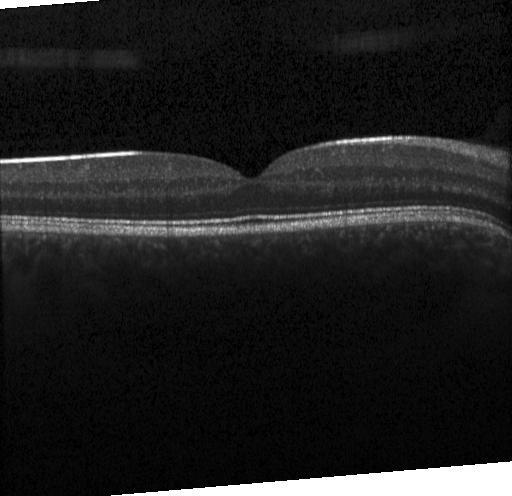
OCT scan showing neither choroidal neovascularization, diabetic macular edema, nor drusen.